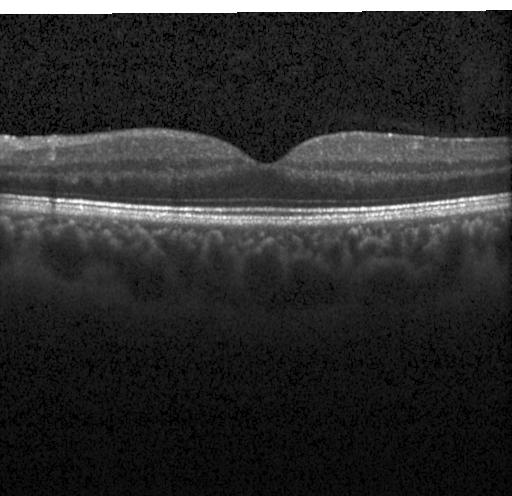 Retinal OCT B-scan.
The scan shows no choroidal neovascularization, diabetic macular edema, or drusen.